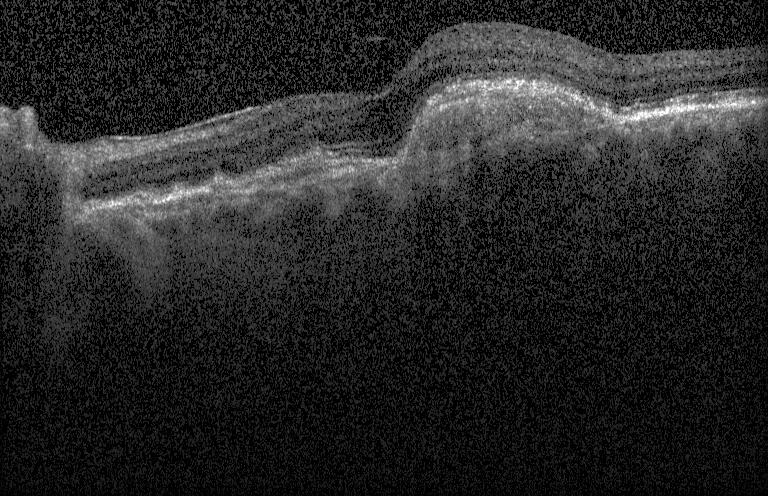

Optical coherence tomography scan, SD-OCT — Macular OCT: a choroidal neovascular membrane.